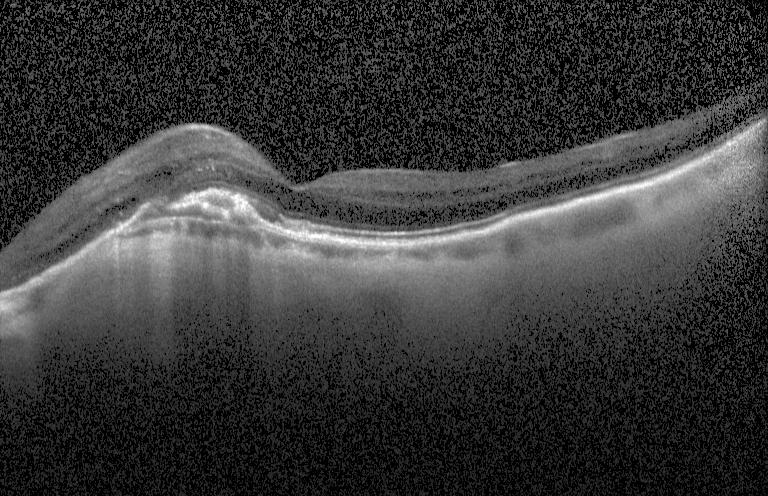
Assessment: choroidal neovascularization.